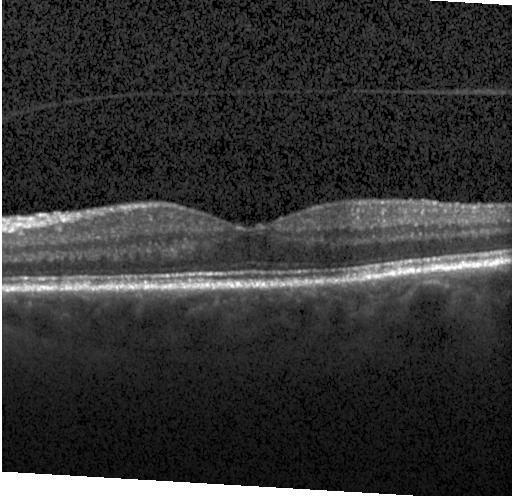

SD-OCT · optical coherence tomography B-scan
Impression: no choroidal neovascularization, diabetic macular edema, or drusen.